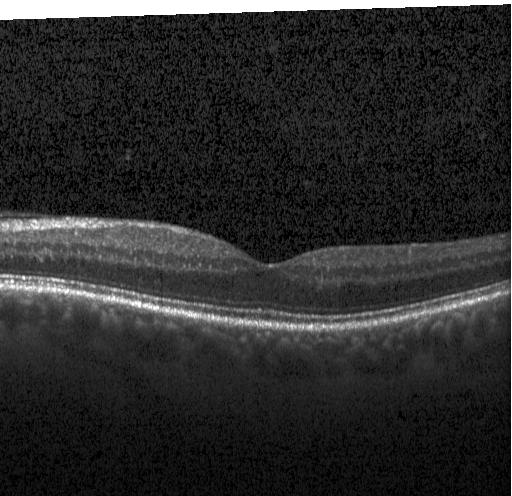
Diagnosis: no evidence of choroidal neovascularization, diabetic macular edema, or drusen.